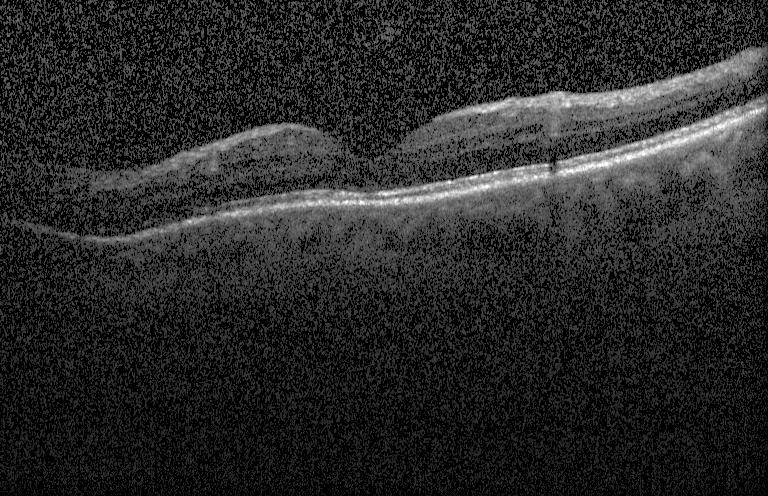
OCT line scan.
Finding: no CNV, no DME, and no drusen.